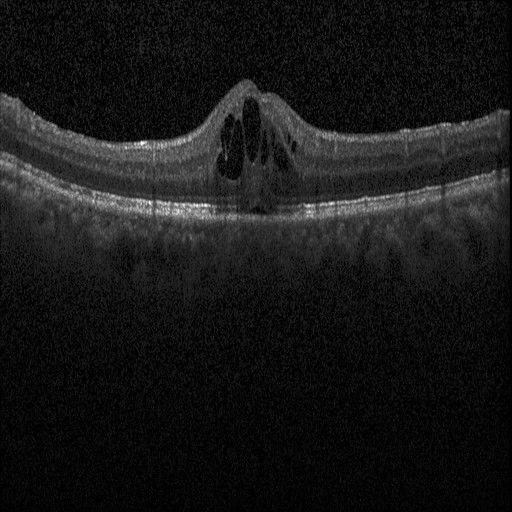

Retinal OCT cross-section. Dx: diabetic macular edema.